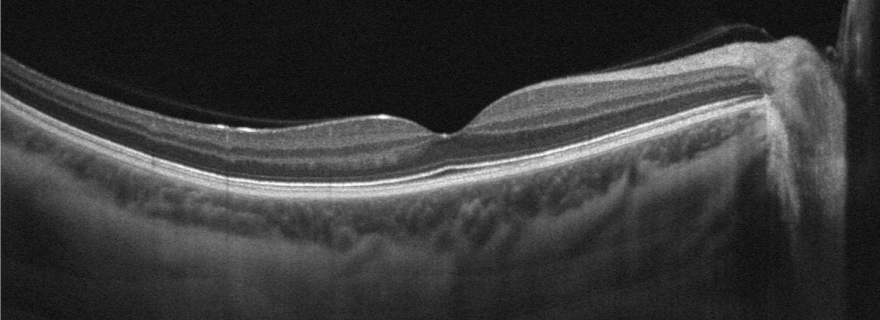 Macular scan · retinal OCT cross-section · instrument: Optovue Avanti RTVue XR. Macular OCT: absence of AMD, DME, ERM, RAO, RVO, and vitreomacular interface disease.